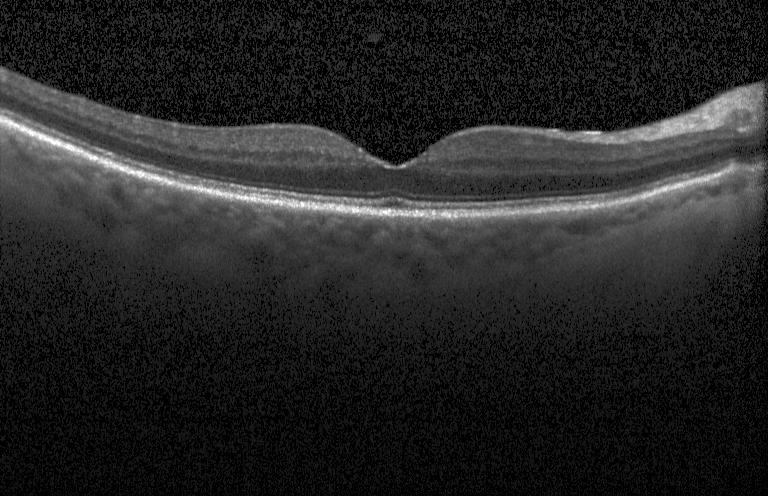
SD-OCT, macular scan, optical coherence tomography scan
Diagnosis: no choroidal neovascularization, no diabetic macular edema, and no drusen.